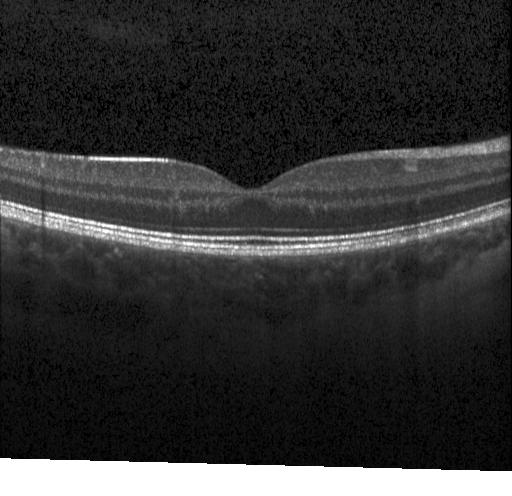 OCT B-scan showing no evidence of choroidal neovascularization, diabetic macular edema, or drusen.